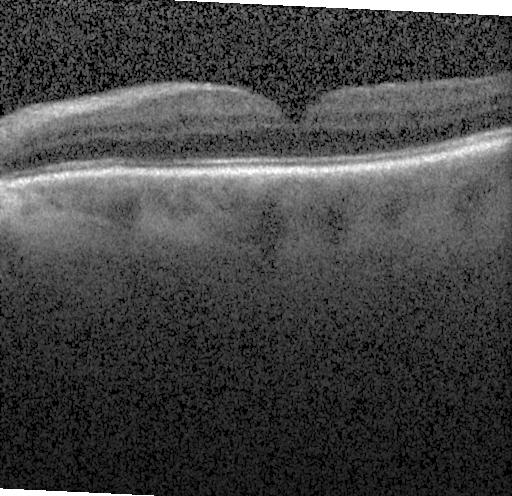 Spectral-domain optical coherence tomography. Retinal OCT cross-section. Acquired on a Heidelberg Spectralis. Horizontal scan through the fovea
Finding: no CNV, no DME, and no drusen.